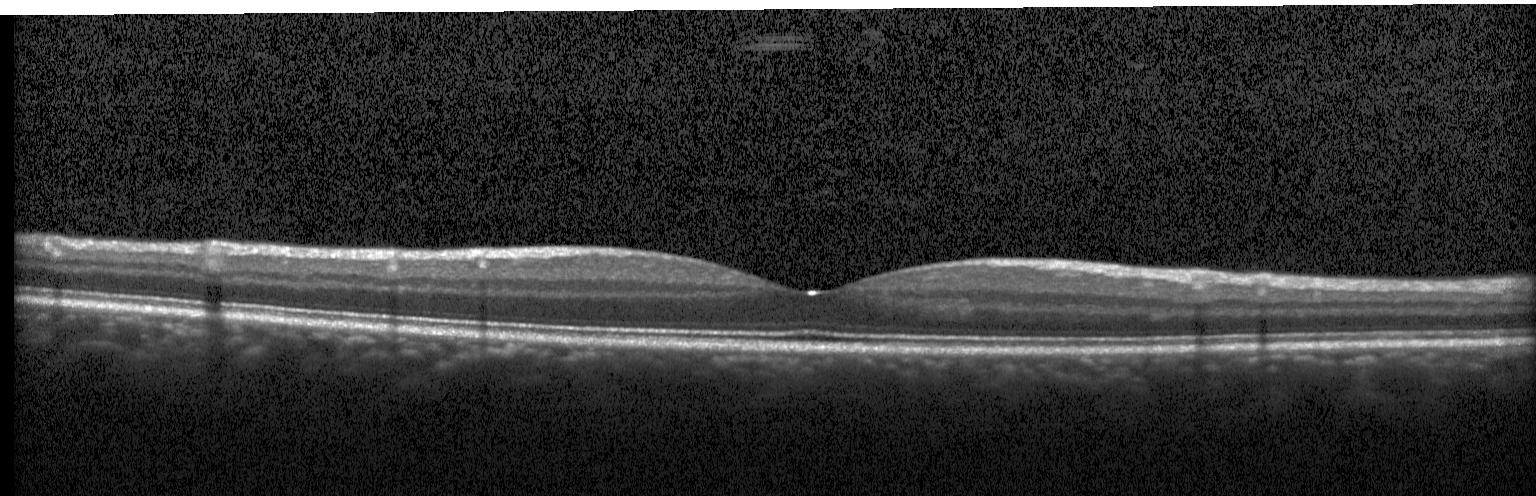
Retinal OCT cross-section. Macular scan. Heidelberg Spectralis OCT system. Spectral-domain OCT.
Dx: no evidence of CNV, DME, or drusen.